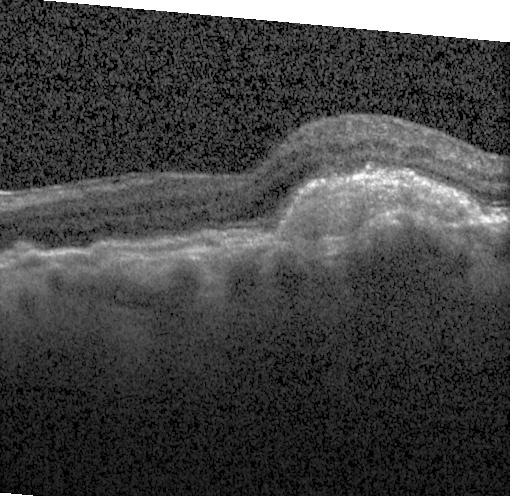
Retinal OCT B-scan
Assessment: a choroidal neovascular membrane.